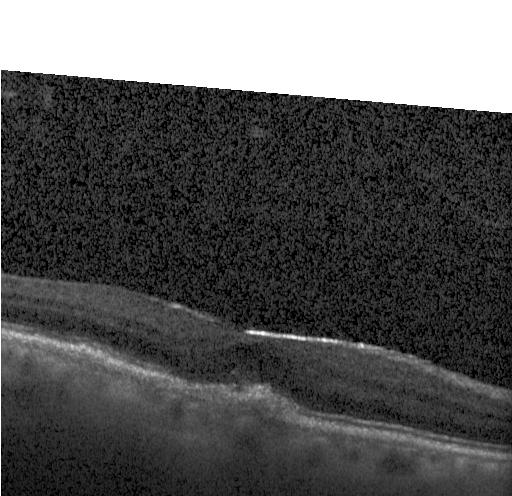 Acquired on a Heidelberg Spectralis. Spectral-domain OCT. OCT B-scan.
Impression: a choroidal neovascular membrane.